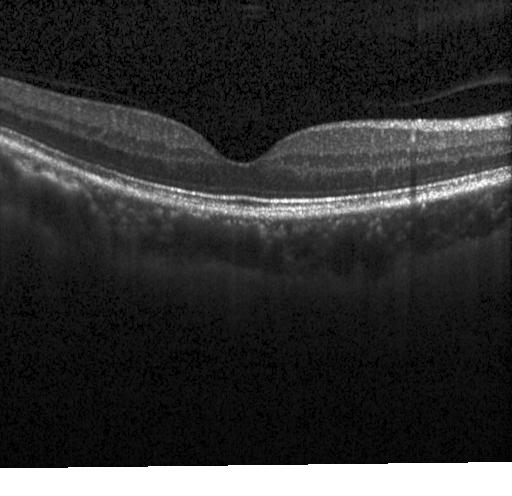 OCT finding: no choroidal neovascularization, diabetic macular edema, or drusen.